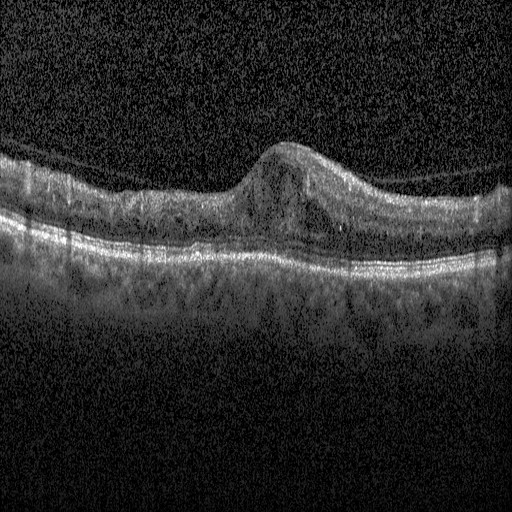
Heidelberg Spectralis OCT system · retinal OCT B-scan · spectral-domain optical coherence tomography — Impression: diabetic macular edema (DME).